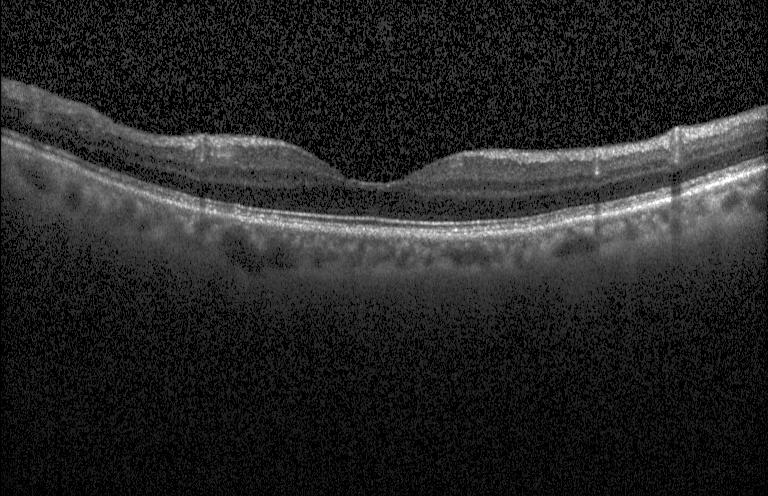

Spectral-domain OCT. Heidelberg Spectralis OCT system. OCT line scan. Macular scan
Impression: no choroidal neovascularization, no diabetic macular edema, and no drusen.